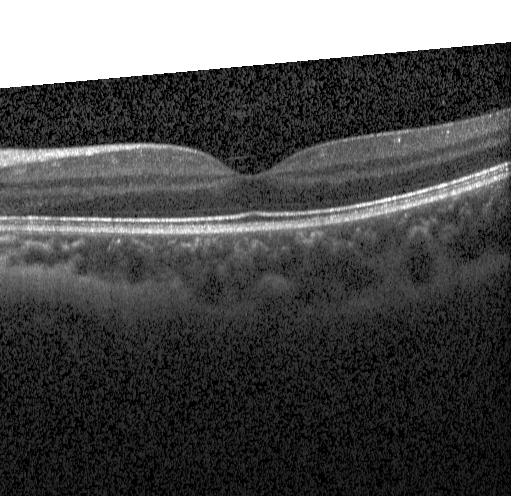

SD-OCT; optical coherence tomography B-scan; acquired on a Heidelberg Spectralis.
No choroidal neovascularization, no diabetic macular edema, and no drusen.